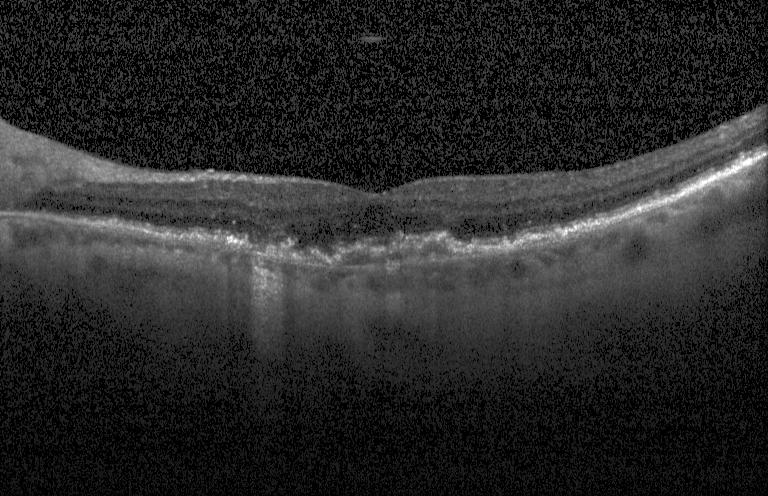
OCT line scan, macular scan, spectral-domain optical coherence tomography. OCT finding: a choroidal neovascular membrane.